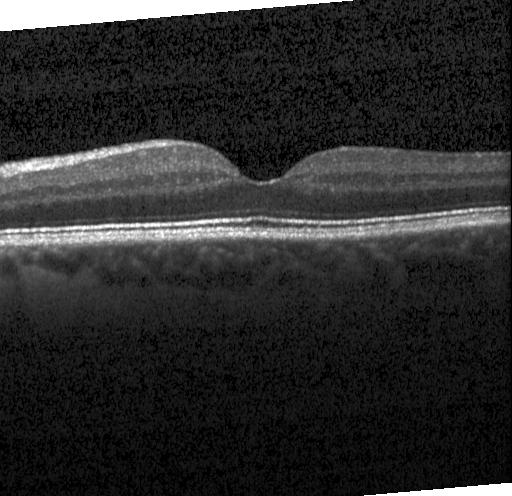

Retinal OCT cross-section. Through the macula. Impression: no choroidal neovascularization, no diabetic macular edema, and no drusen.